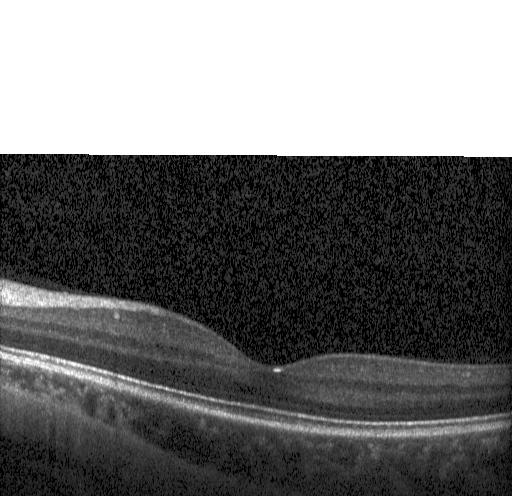

Spectral-domain OCT B-scan: no CNV, DME, or drusen.